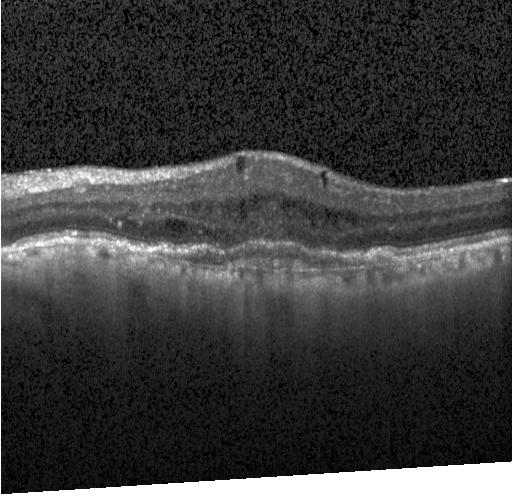
OCT B-scan. Diagnosis: choroidal neovascularization (CNV).